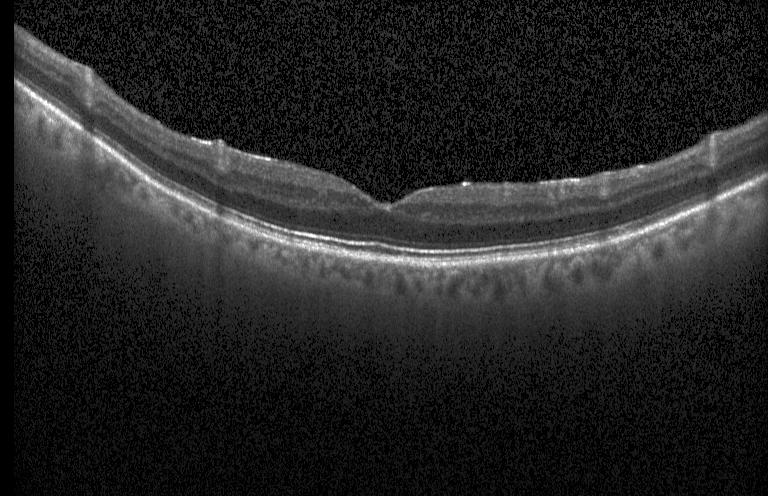 SD-OCT, Heidelberg Spectralis, centered on the fovea, optical coherence tomography scan — Assessment: no choroidal neovascularization, diabetic macular edema, or drusen.